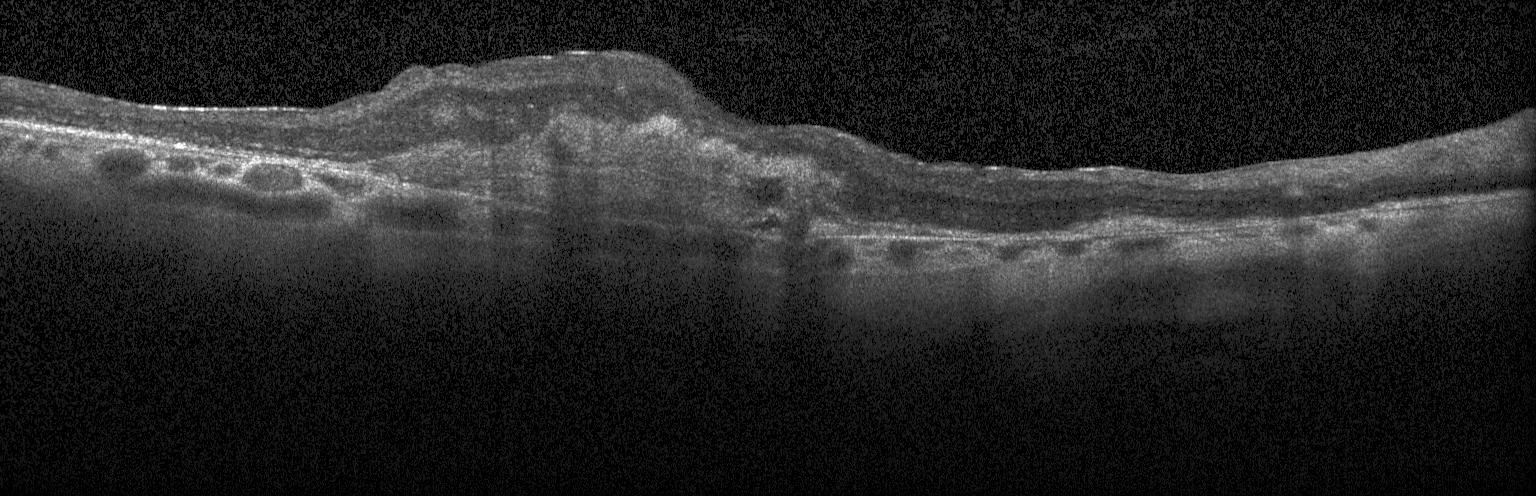
This B-scan demonstrates CNV.